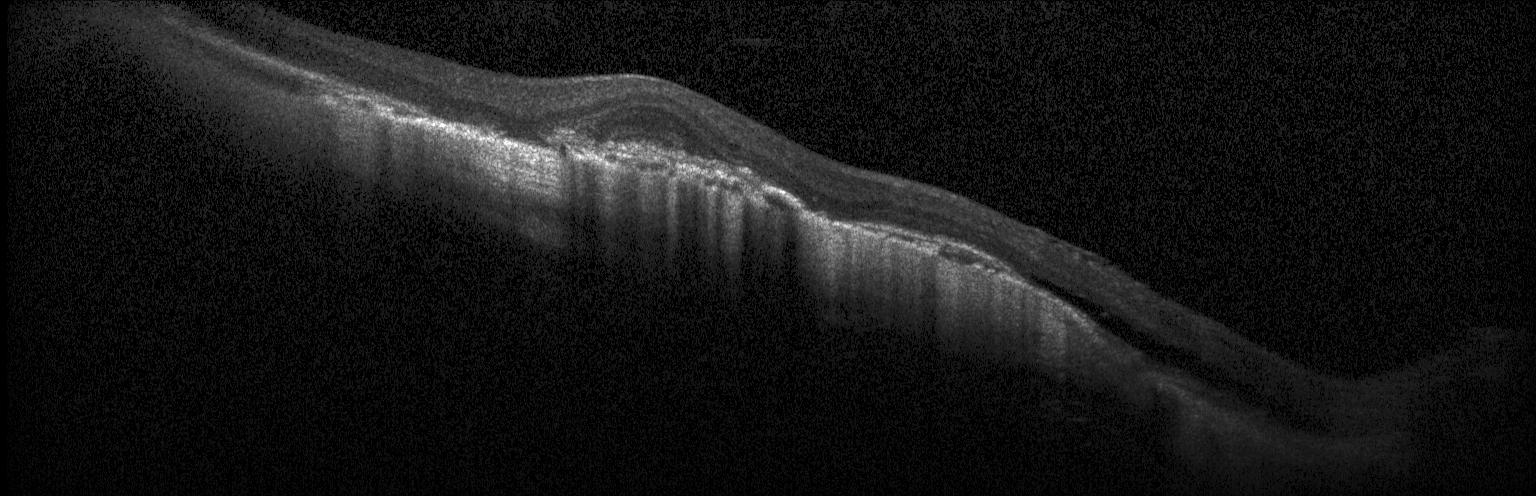 The scan shows a choroidal neovascular membrane.